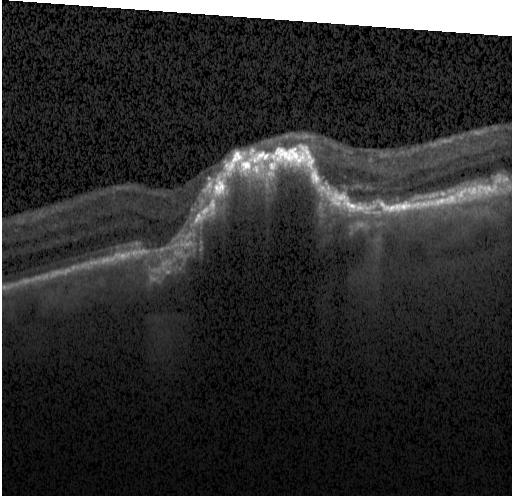

Macular OCT: choroidal neovascularization.